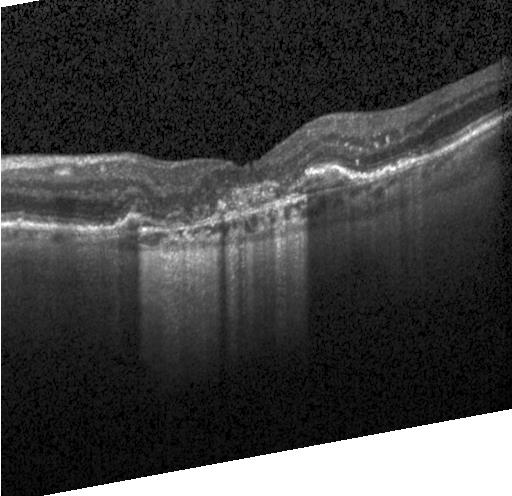

This B-scan demonstrates a choroidal neovascular membrane.